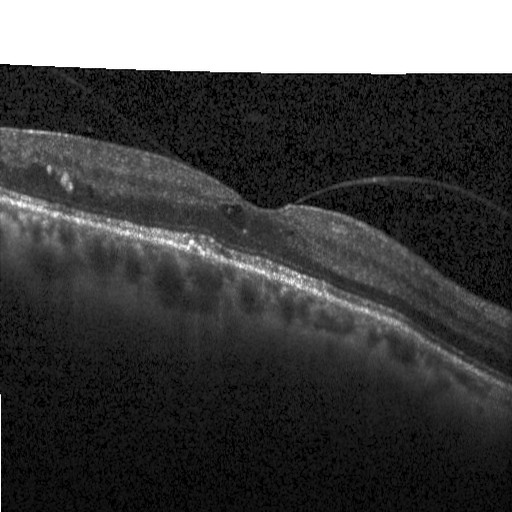
OCT line scan · centered on the fovea · instrument: Heidelberg Spectralis · spectral-domain optical coherence tomography
This B-scan demonstrates diabetic macular edema.